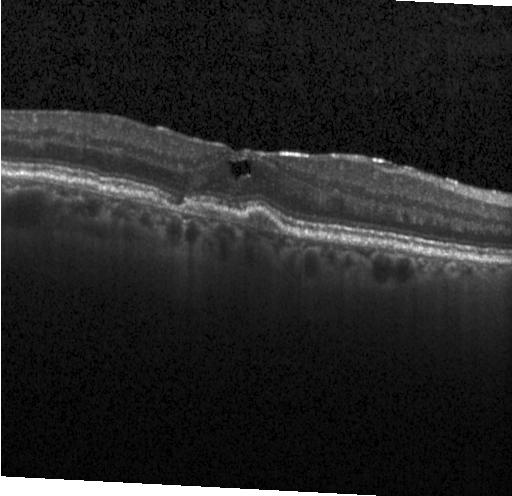
Spectral-domain optical coherence tomography. Horizontal scan through the fovea. Retinal OCT cross-section.
The scan shows a choroidal neovascular membrane.